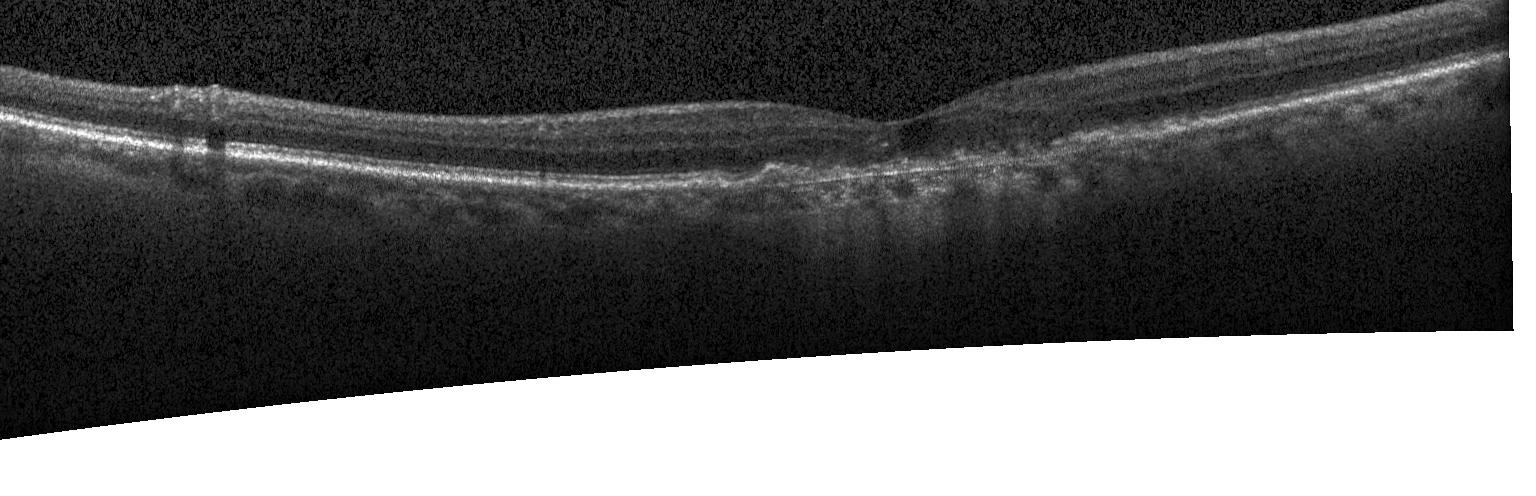 Diagnosis: a choroidal neovascular membrane.